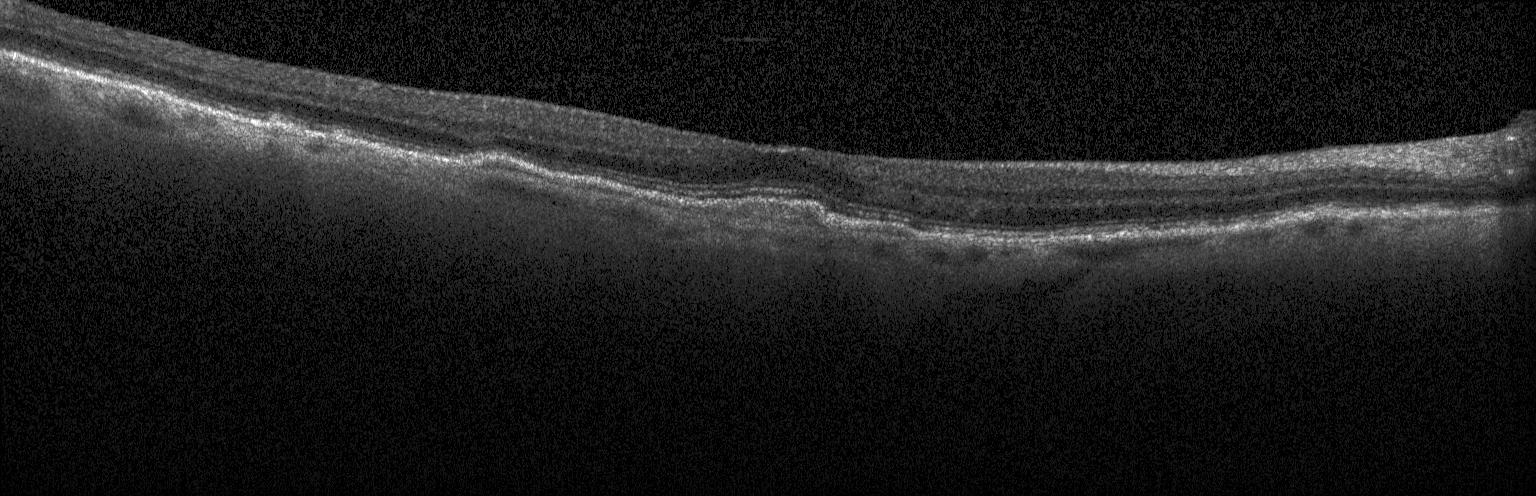 This B-scan demonstrates a choroidal neovascular membrane.